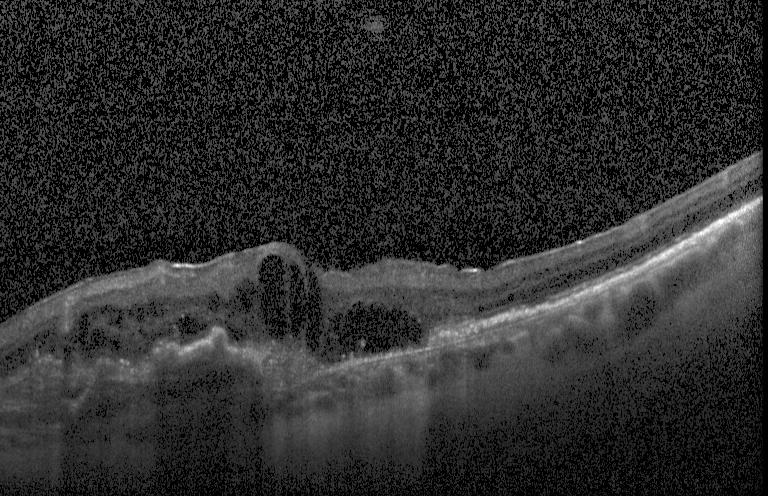 Dx: choroidal neovascularization (CNV).